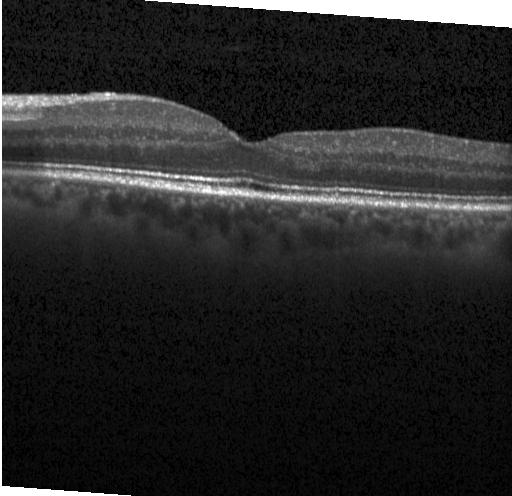
Retinal OCT cross-section
Macular OCT: no choroidal neovascularization, no diabetic macular edema, and no drusen.